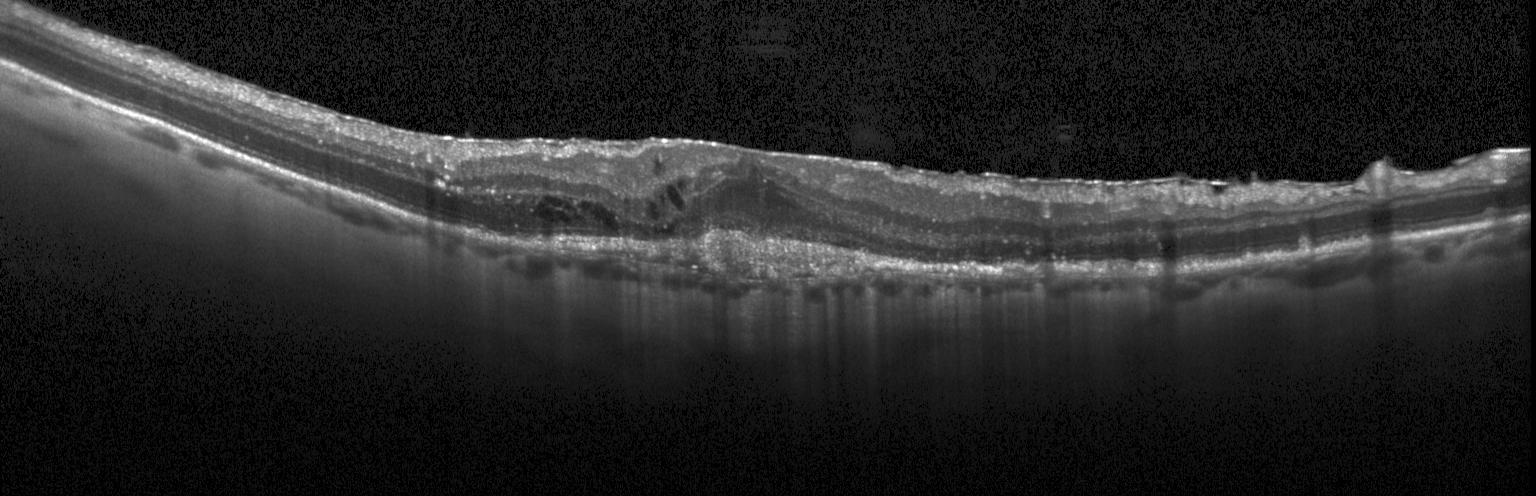 Through the macula; optical coherence tomography B-scan. Finding: choroidal neovascularization.